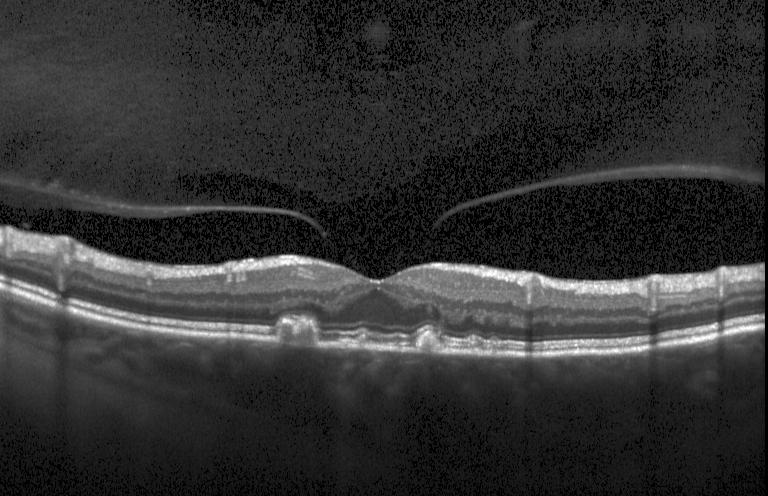
Optical coherence tomography B-scan
Macular OCT: sub-RPE drusenoid deposits.